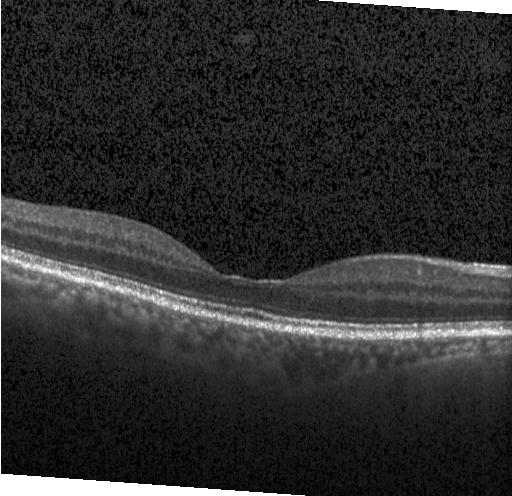 Optical coherence tomography scan, fovea-centered, Heidelberg Spectralis OCT system. Dx: no CNV, DME, or drusen.